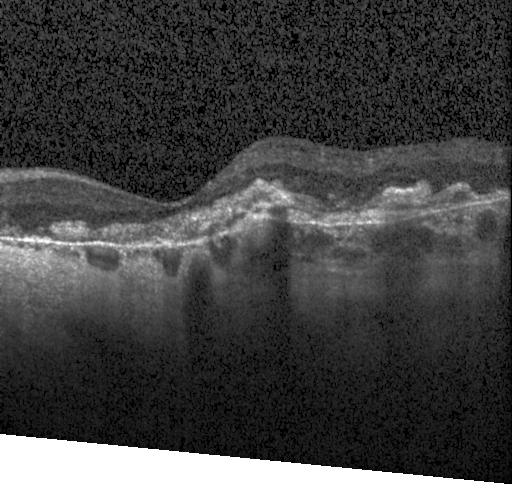 OCT B-scan — Macular OCT: a choroidal neovascular membrane.